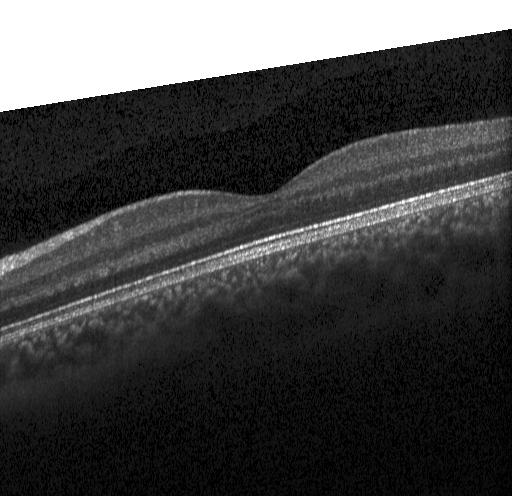

Diagnosis: no evidence of CNV, DME, or drusen.